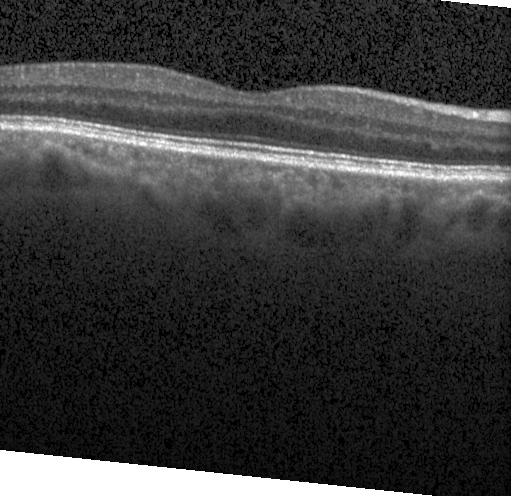 Horizontal scan through the fovea · retinal OCT cross-section
Macular OCT: no choroidal neovascularization, no diabetic macular edema, and no drusen.